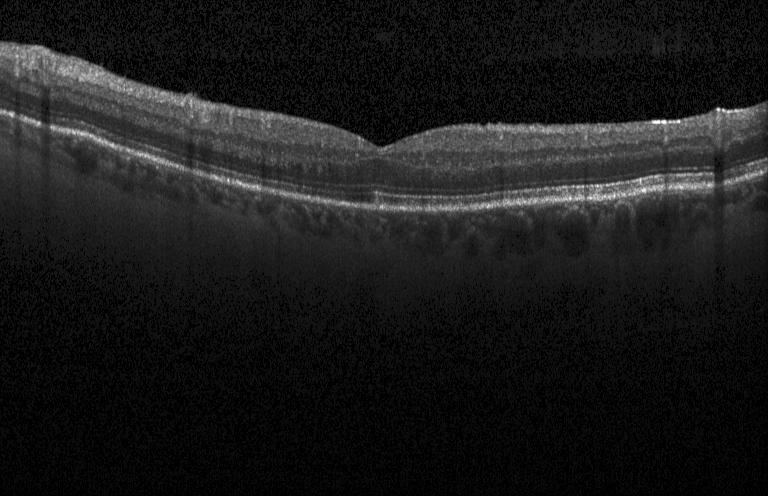
Finding: no choroidal neovascularization, no diabetic macular edema, and no drusen.